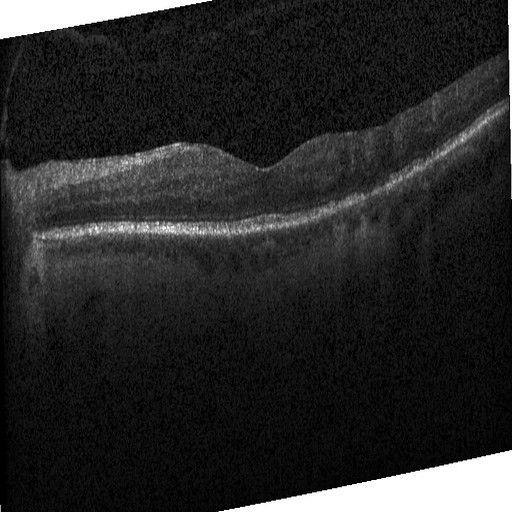
Spectral-domain optical coherence tomography. Acquired on a Heidelberg Spectralis. Retinal OCT B-scan
Assessment: DME.